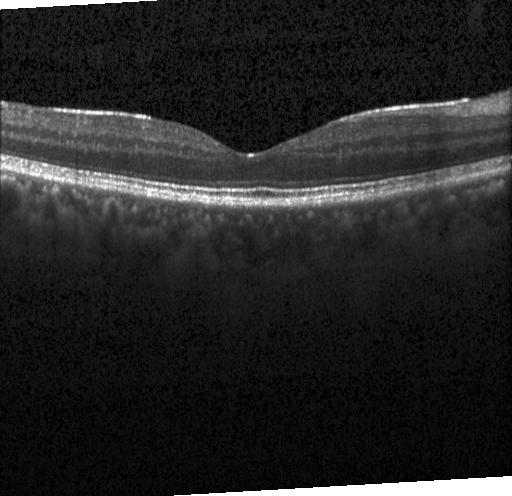
Retinal OCT cross-section, Heidelberg Spectralis OCT system, fovea-centered, SD-OCT — OCT finding: no choroidal neovascularization, diabetic macular edema, or drusen.